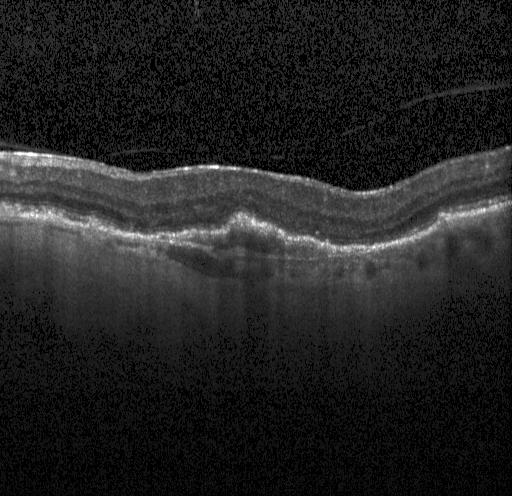 Choroidal neovascularization (CNV).